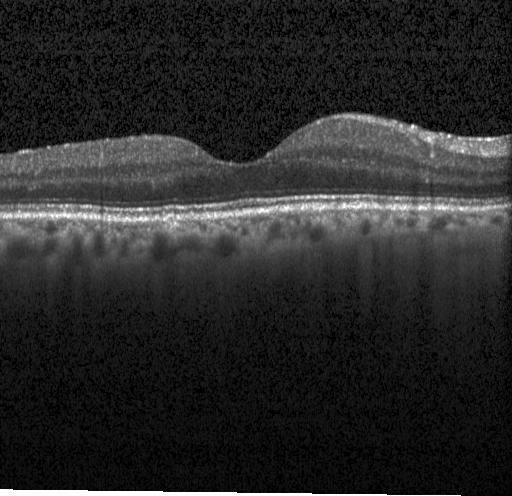 OCT B-scan showing no CNV, no DME, and no drusen.